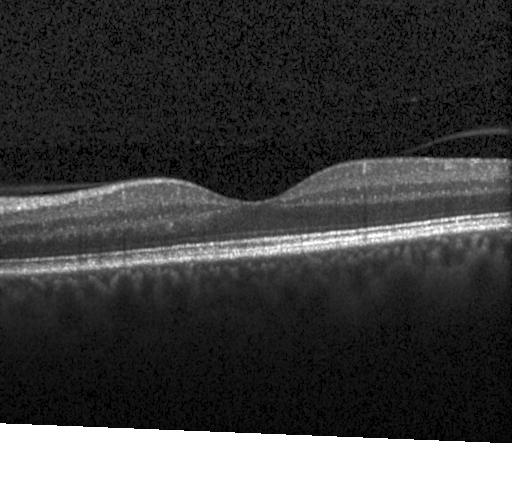 OCT finding: no evidence of CNV, DME, or drusen.